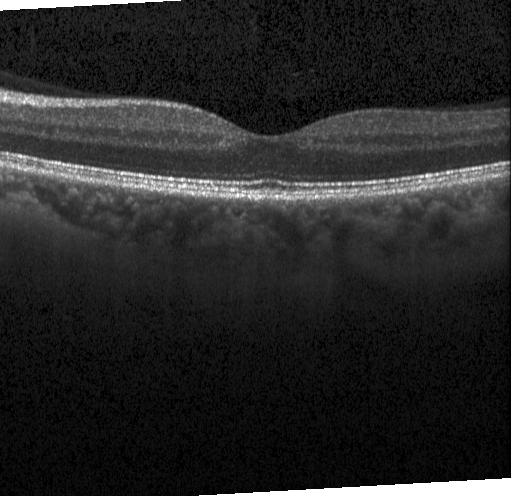

Macular OCT demonstrating no choroidal neovascularization, no diabetic macular edema, and no drusen.